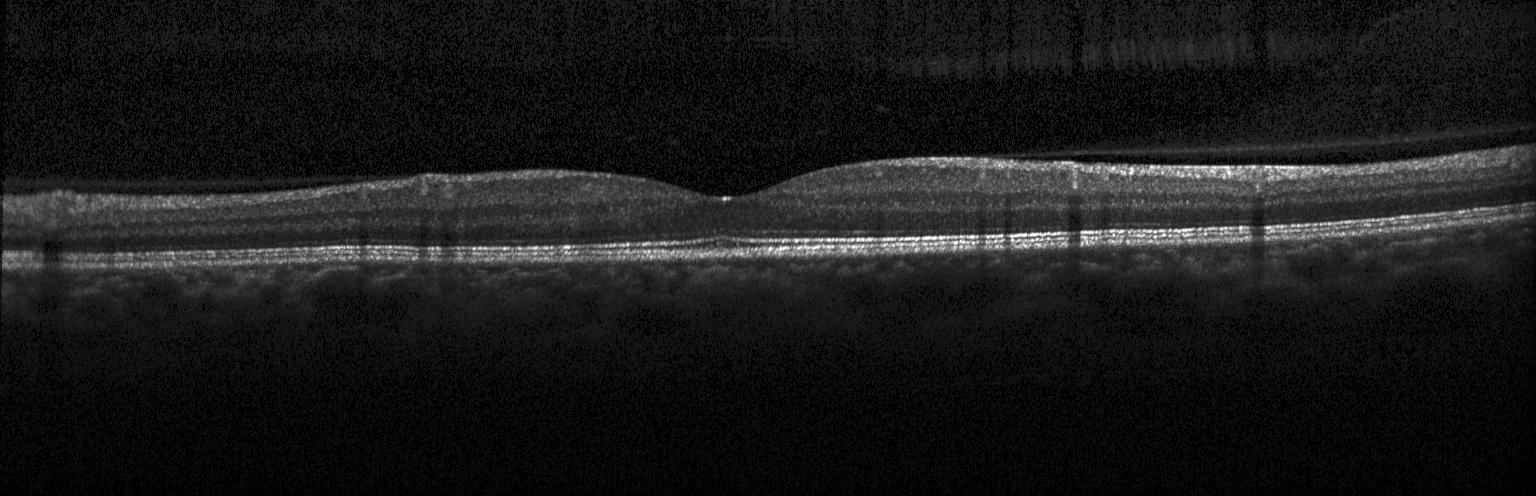

Retinal OCT cross-section. SD-OCT. Horizontal scan through the fovea.
Impression: no choroidal neovascularization, no diabetic macular edema, and no drusen.